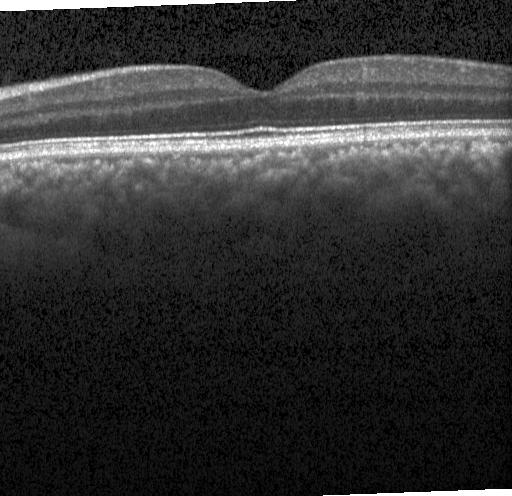

OCT B-scan showing no choroidal neovascularization, diabetic macular edema, or drusen.